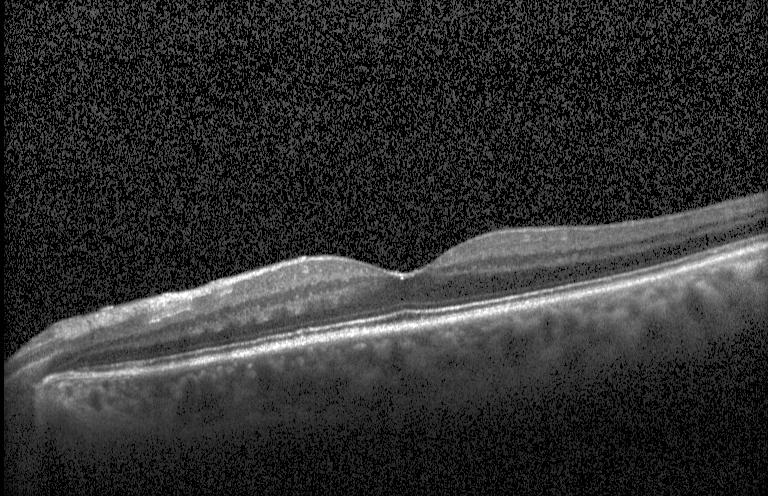

Dx: no choroidal neovascularization, no diabetic macular edema, and no drusen.